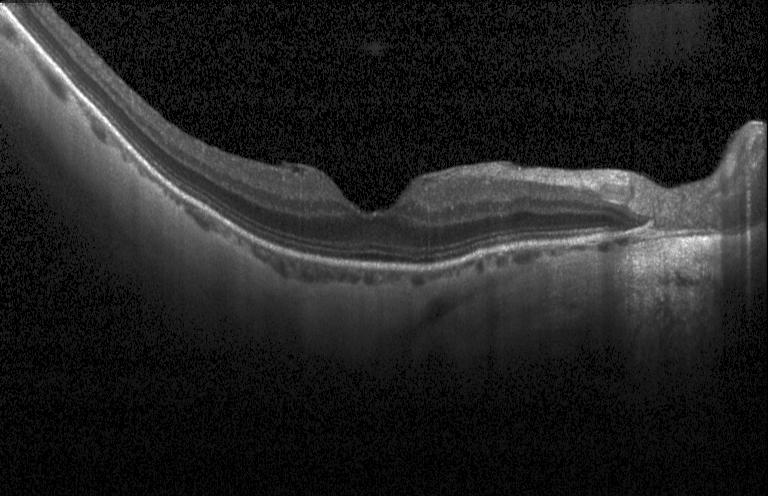
Macular OCT: neither CNV, DME, nor drusen.